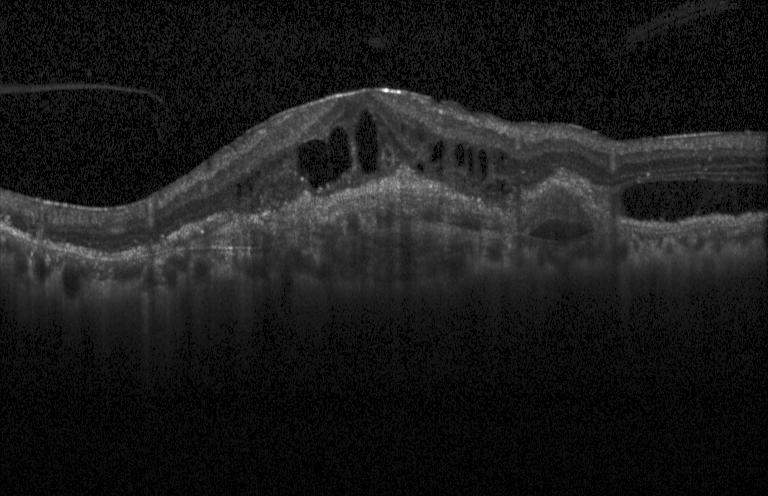
Macular scan. Retinal OCT B-scan. SD-OCT
The scan shows a choroidal neovascular membrane.